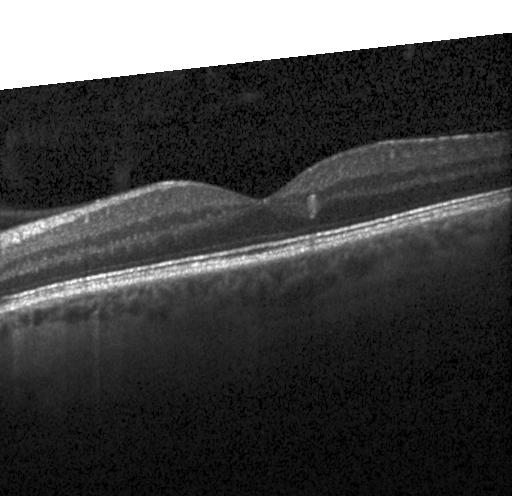 Retinal OCT cross-section, Heidelberg Spectralis OCT system, SD-OCT — This B-scan demonstrates no choroidal neovascularization, diabetic macular edema, or drusen.